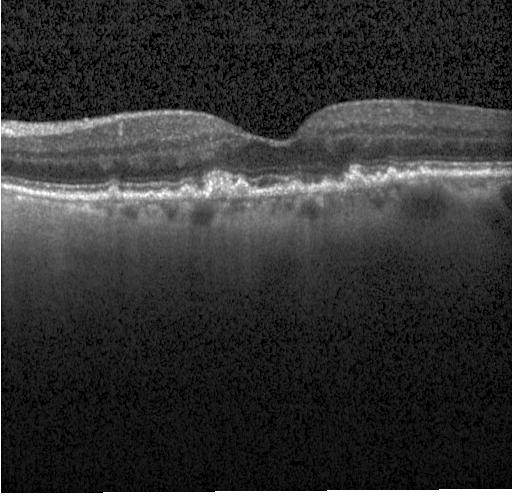
Spectral-domain OCT. Centered on the fovea. Optical coherence tomography B-scan
Finding: drusen.